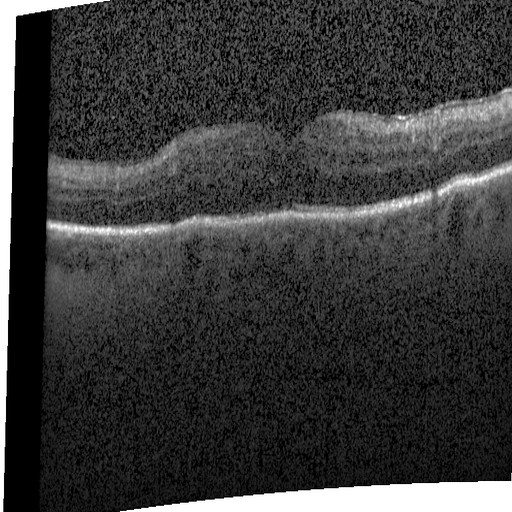 Optical coherence tomography B-scan.
Assessment: diabetic macular edema (DME).